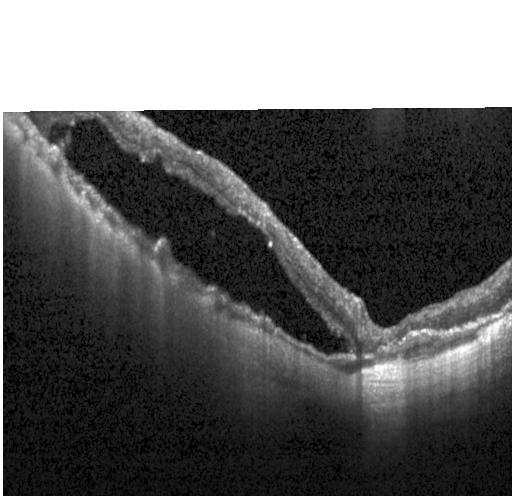

Spectral-domain OCT B-scan: choroidal neovascularization.